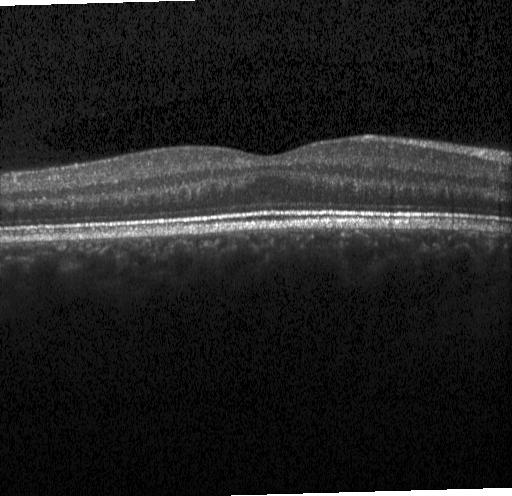
Retinal OCT cross-section. Impression: no choroidal neovascularization, no diabetic macular edema, and no drusen.